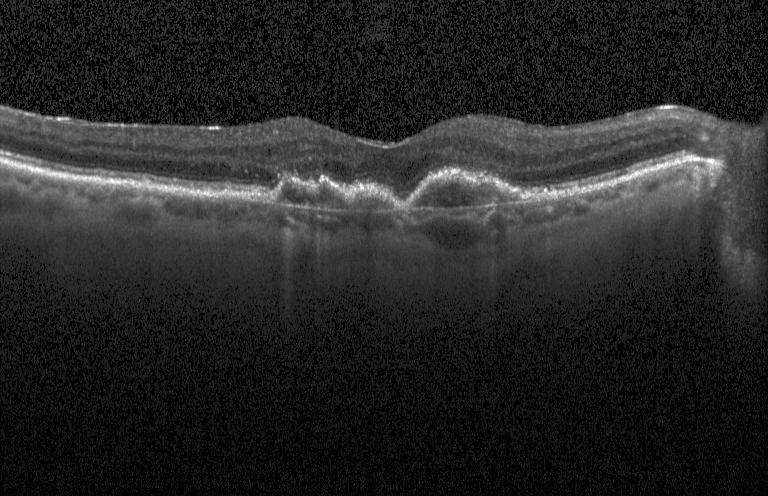
Dx: a choroidal neovascular membrane.